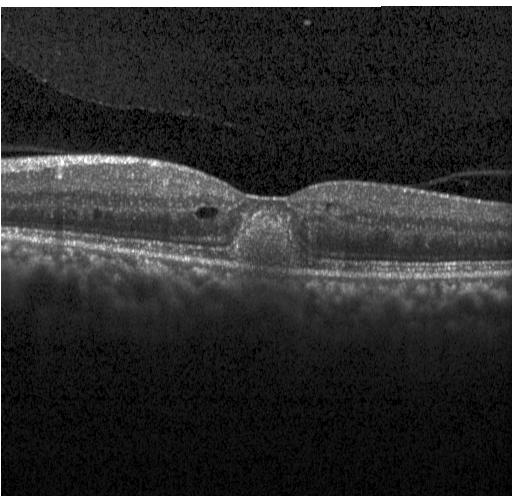

OCT B-scan — A choroidal neovascular membrane.